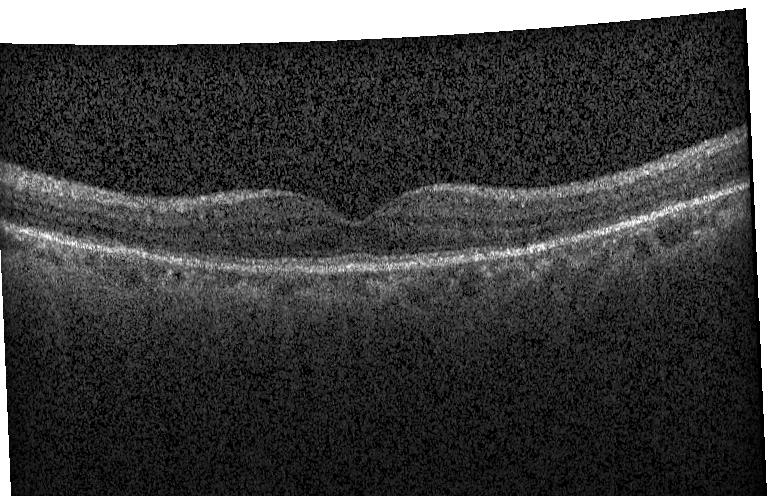

Optical coherence tomography scan · instrument: Heidelberg Spectralis. Macular OCT: no CNV, no DME, and no drusen.